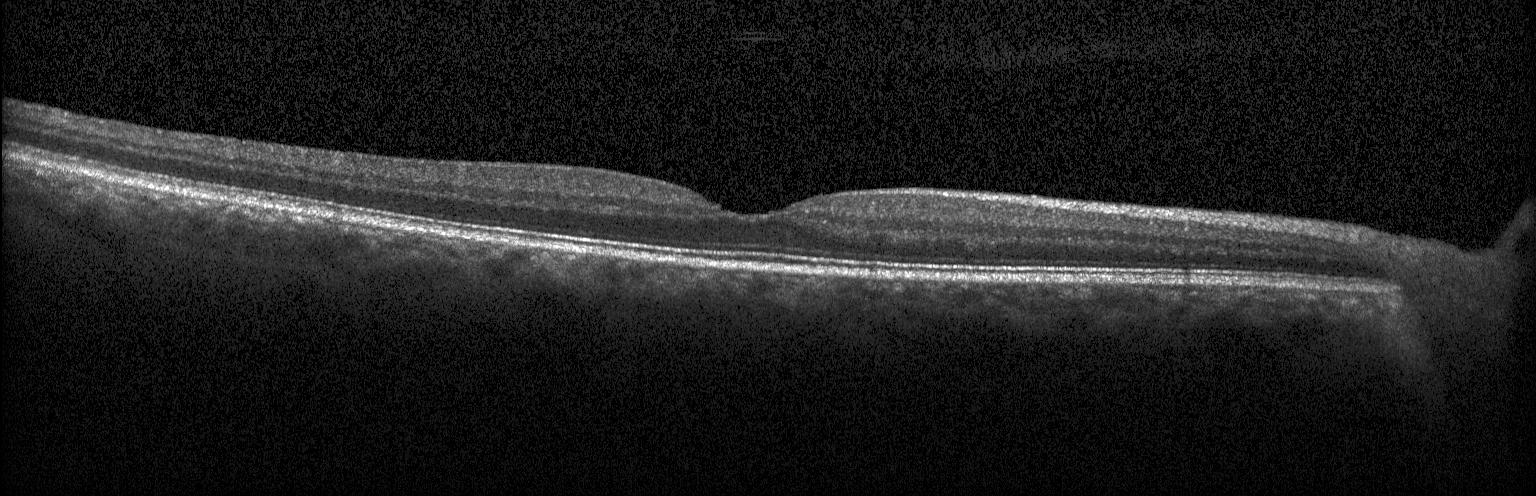
Neither choroidal neovascularization, diabetic macular edema, nor drusen.